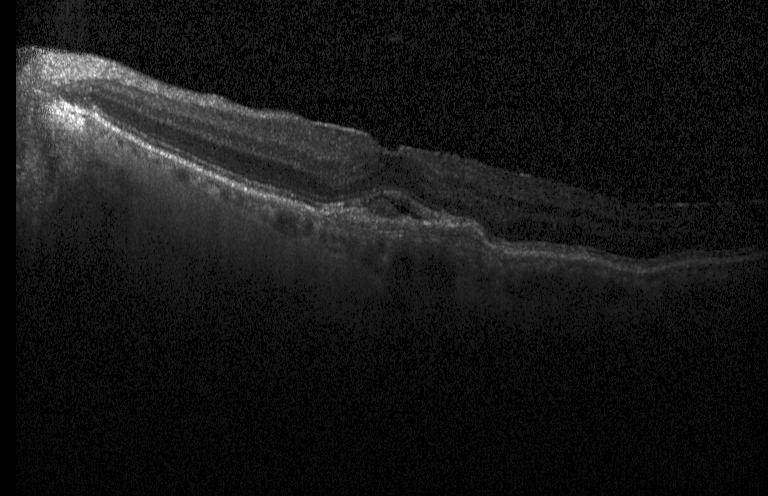

Impression: choroidal neovascularization (CNV).